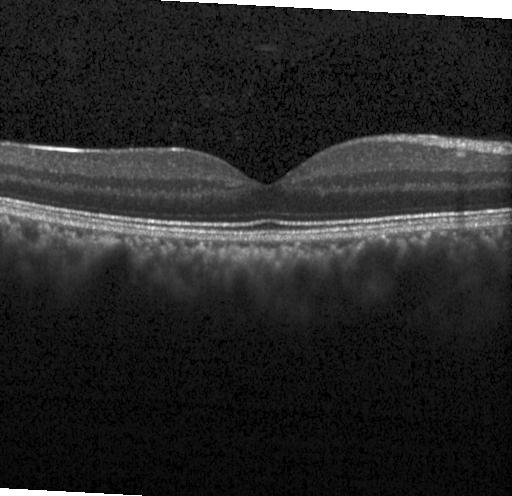
SD-OCT · macular scan · OCT B-scan · acquired on a Heidelberg Spectralis.
Dx: no evidence of CNV, DME, or drusen.